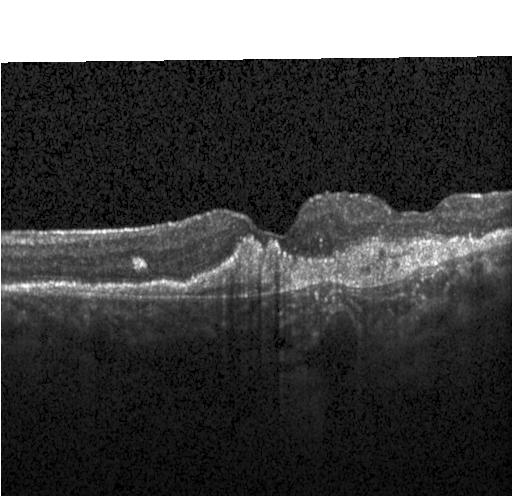
Macular OCT demonstrating CNV.